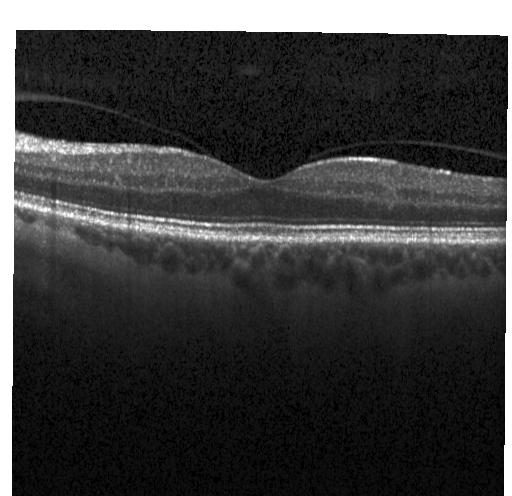 Heidelberg Spectralis. Fovea-centered. OCT line scan. Spectral-domain optical coherence tomography. OCT finding: neither choroidal neovascularization, diabetic macular edema, nor drusen.